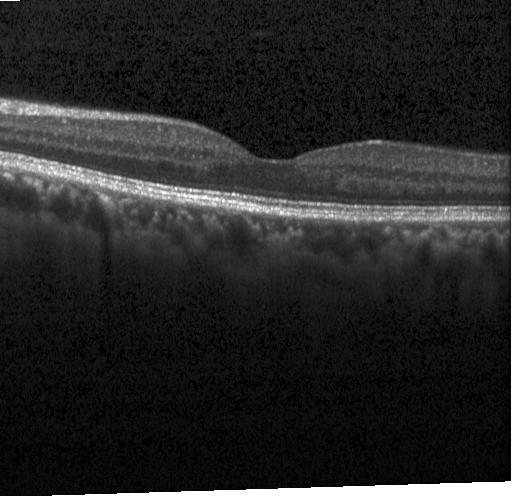

Impression: no choroidal neovascularization, no diabetic macular edema, and no drusen.